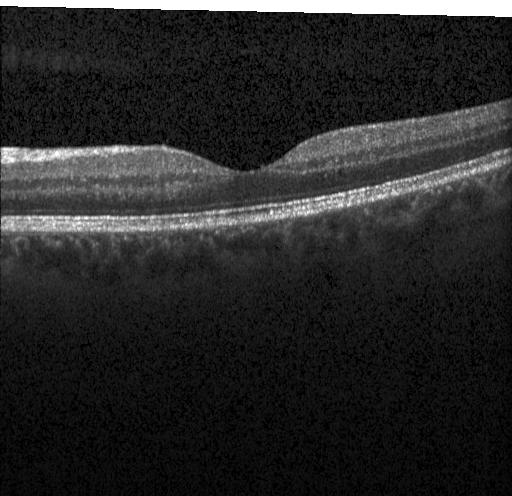

Optical coherence tomography scan
This B-scan demonstrates neither CNV, DME, nor drusen.